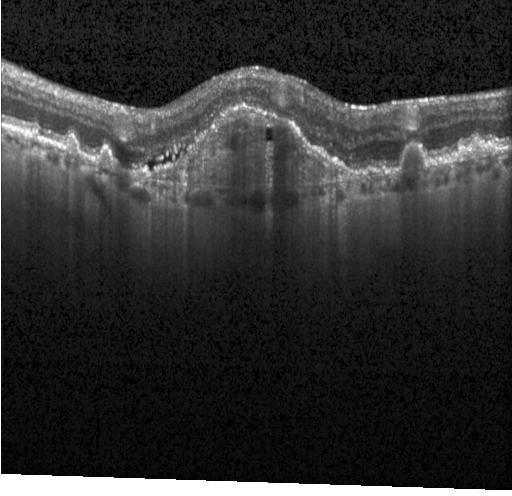

Spectral-domain OCT. Fovea-centered. Instrument: Heidelberg Spectralis. Optical coherence tomography B-scan
This B-scan demonstrates a choroidal neovascular membrane.